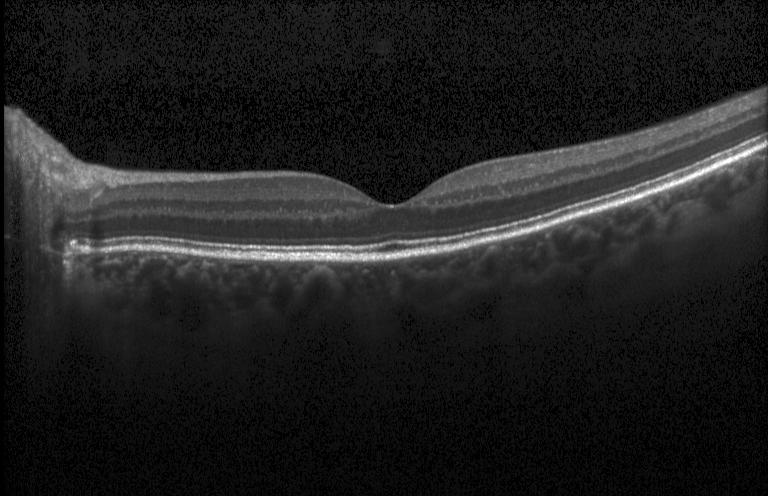 Optical coherence tomography scan.
This B-scan demonstrates no choroidal neovascularization, no diabetic macular edema, and no drusen.